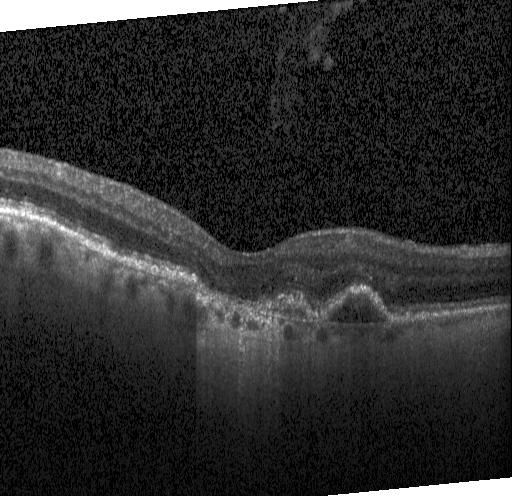
Retinal OCT B-scan. Diagnosis: choroidal neovascularization (CNV).